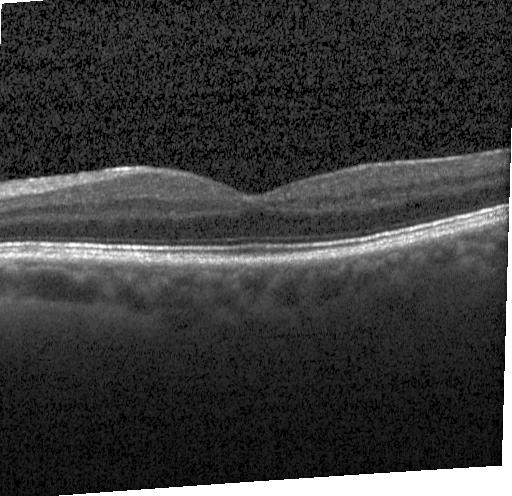

Macular scan, acquired on a Heidelberg Spectralis, retinal OCT B-scan, spectral-domain optical coherence tomography.
Assessment: no choroidal neovascularization, no diabetic macular edema, and no drusen.